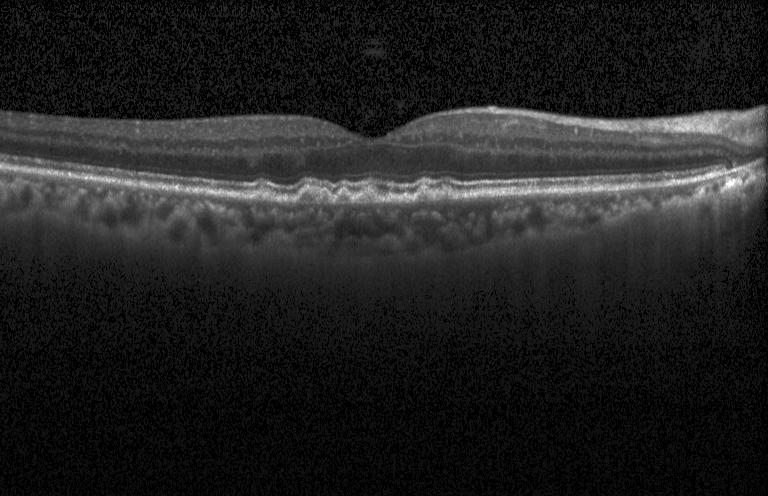
OCT scan showing multiple drusen.